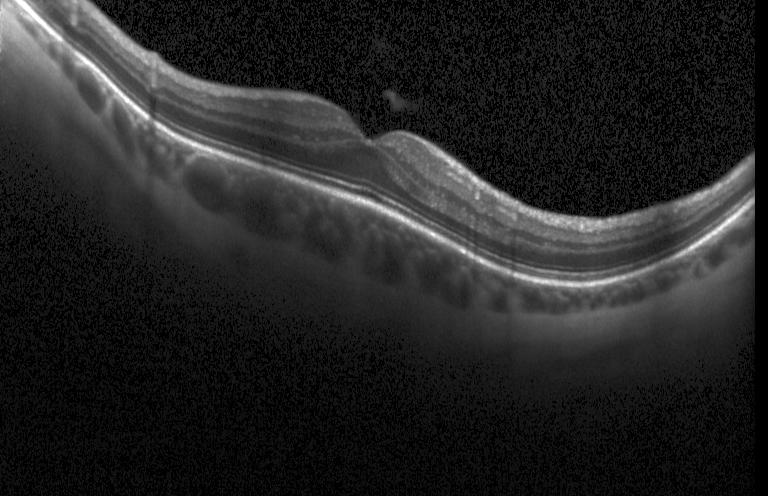

Impression: no choroidal neovascularization, diabetic macular edema, or drusen.